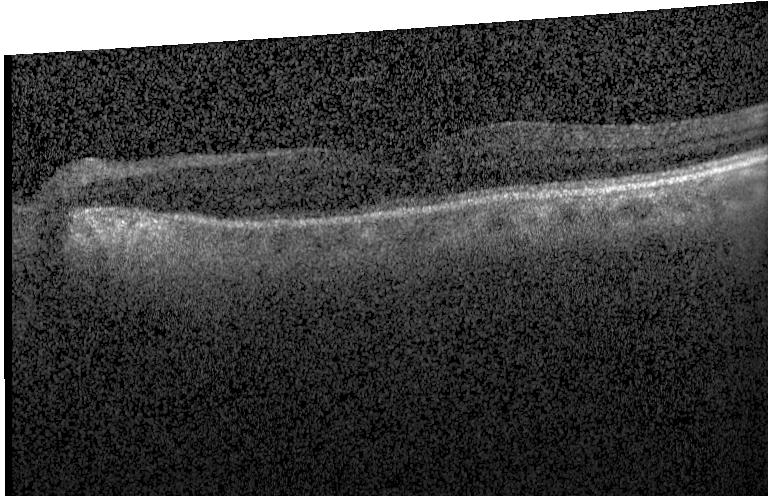

Finding: no CNV, no DME, and no drusen.